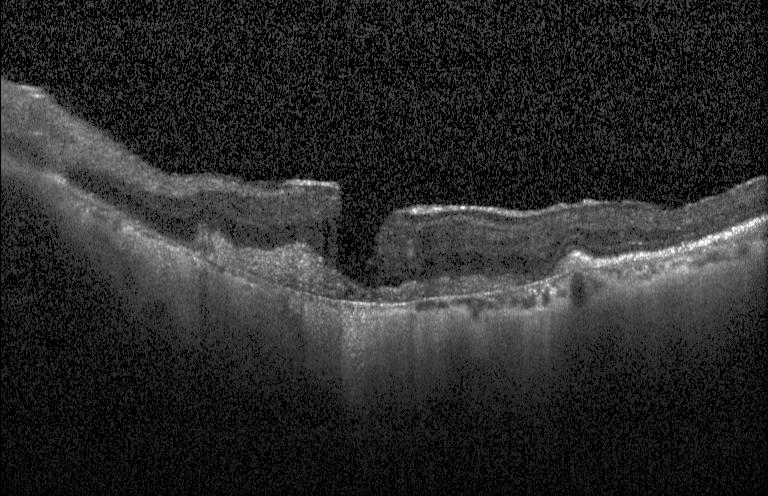 Diagnosis: a choroidal neovascular membrane.